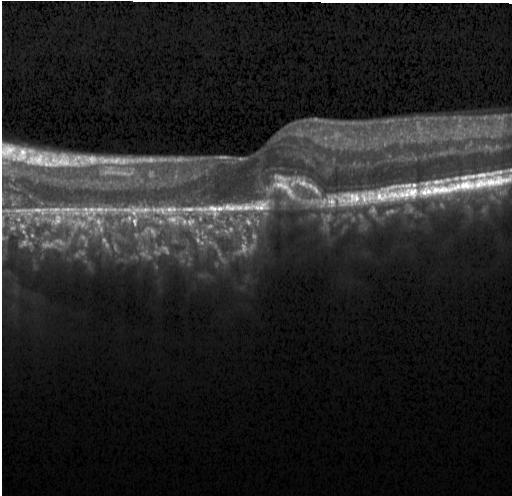 Centered on the fovea · instrument: Heidelberg Spectralis · spectral-domain optical coherence tomography · OCT B-scan — Diagnosis: a choroidal neovascular membrane.